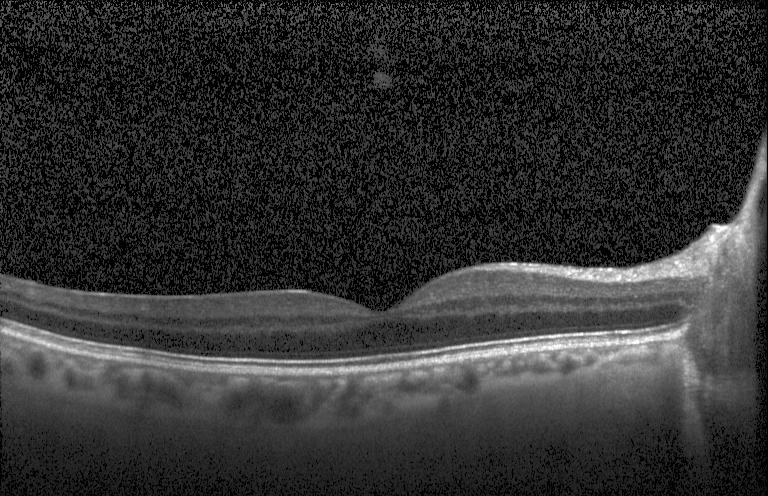

Assessment: neither CNV, DME, nor drusen.